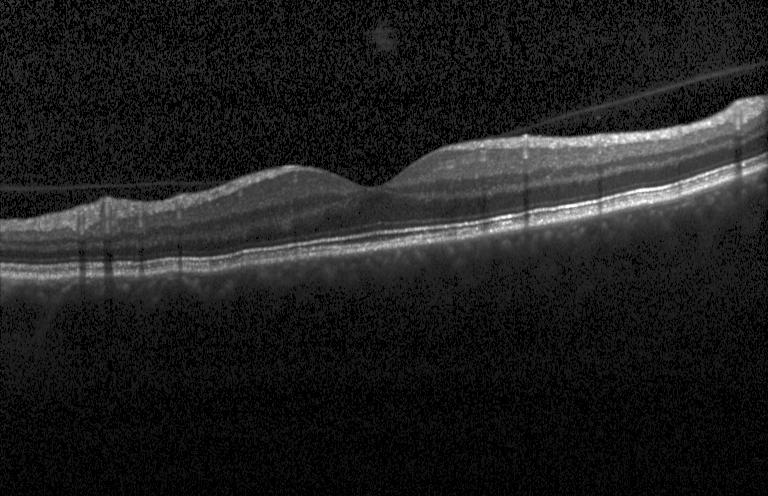 OCT B-scan — Finding: no evidence of choroidal neovascularization, diabetic macular edema, or drusen.